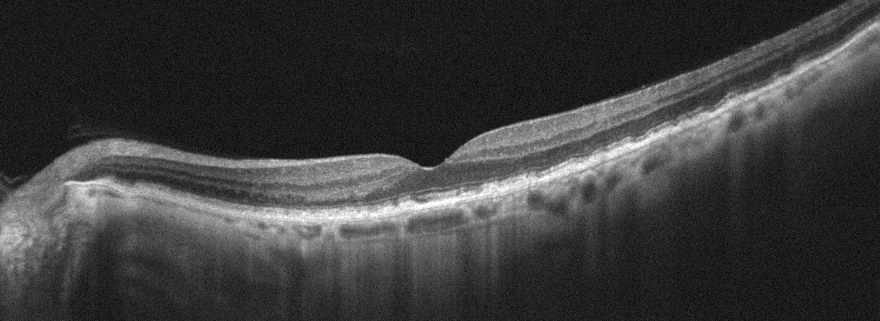
Assessment: AMD.